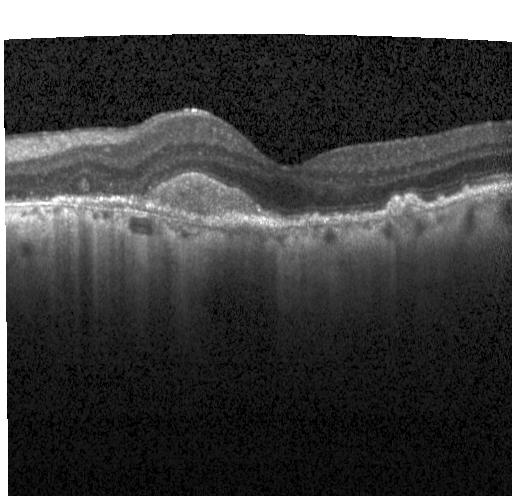
Optical coherence tomography scan. Macular OCT: choroidal neovascularization.